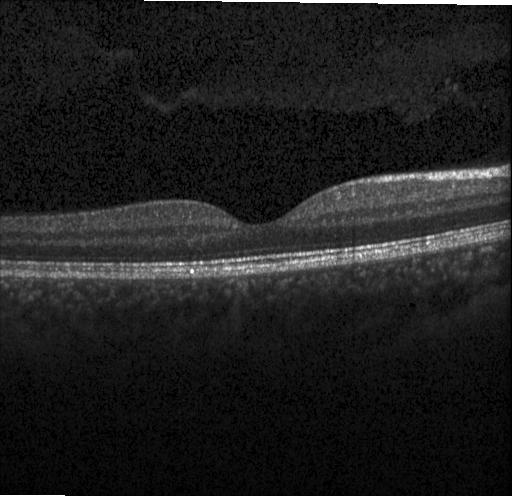

The scan shows no evidence of choroidal neovascularization, diabetic macular edema, or drusen.